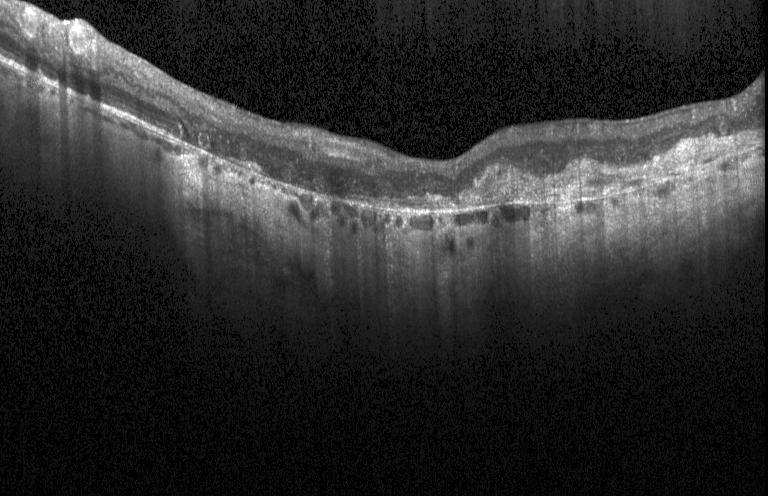

Finding: choroidal neovascularization.